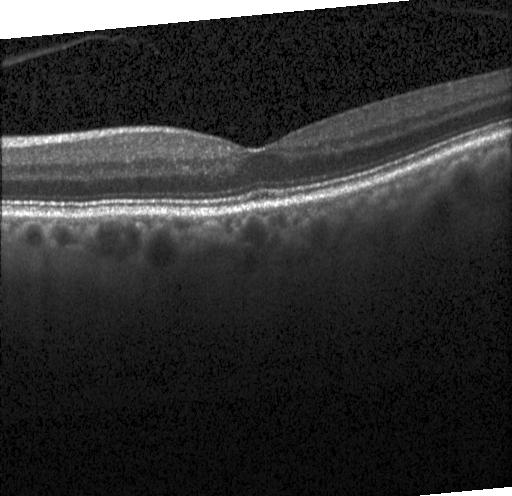 Centered on the fovea; spectral-domain OCT; instrument: Heidelberg Spectralis; optical coherence tomography B-scan — The scan shows neither CNV, DME, nor drusen.